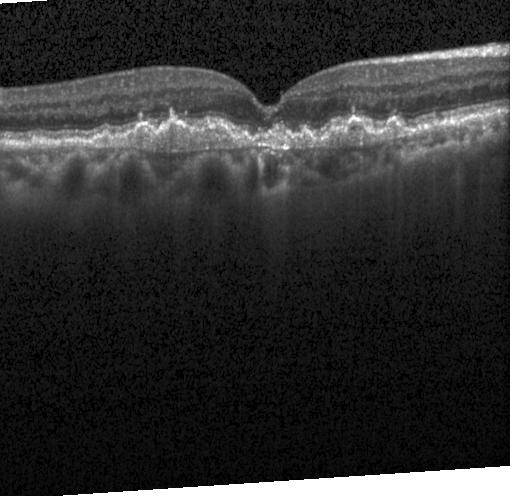 Optical coherence tomography B-scan — Impression: a choroidal neovascular membrane.